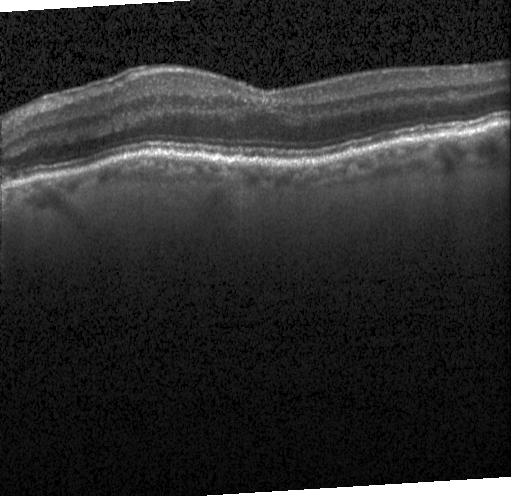 Spectral-domain optical coherence tomography; optical coherence tomography B-scan — Finding: no CNV, DME, or drusen.